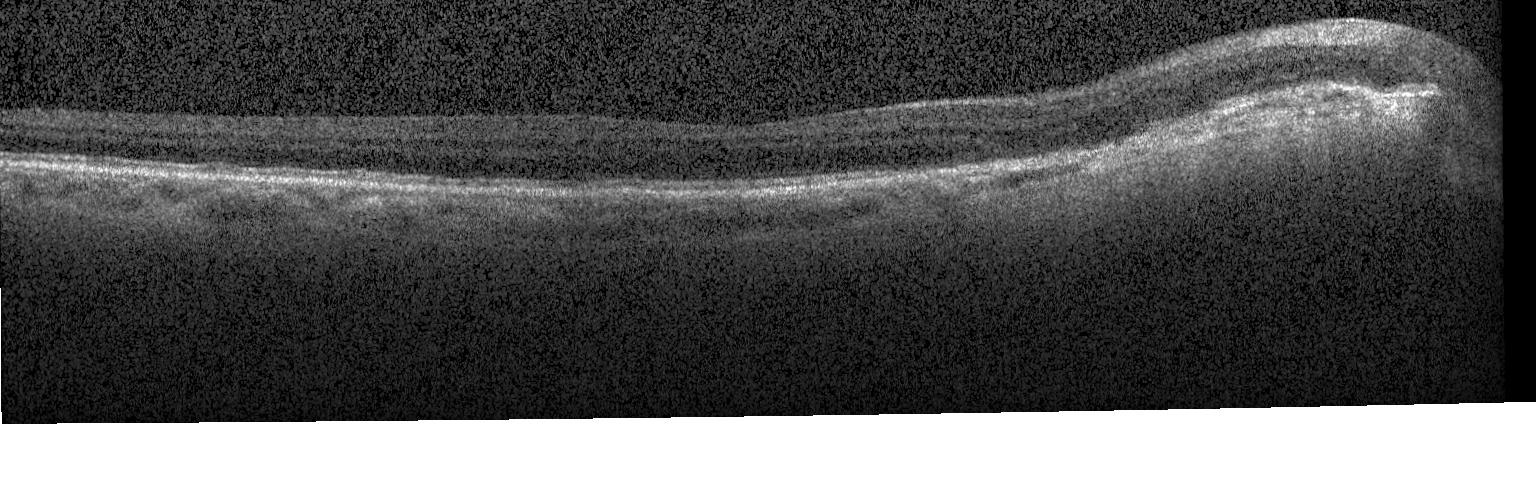
Spectral-domain OCT. Retinal OCT B-scan. Diagnosis: choroidal neovascularization (CNV).